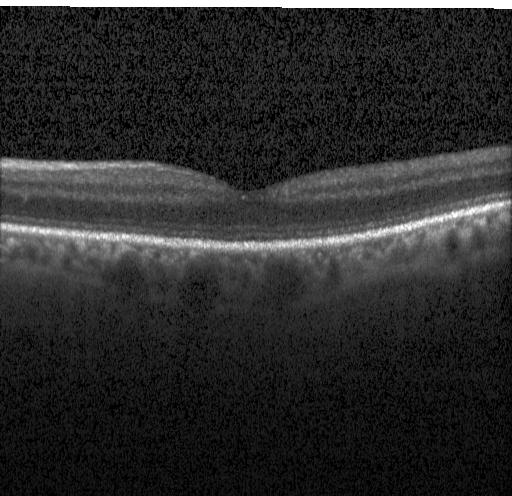

OCT B-scan.
The scan shows no CNV, no DME, and no drusen.